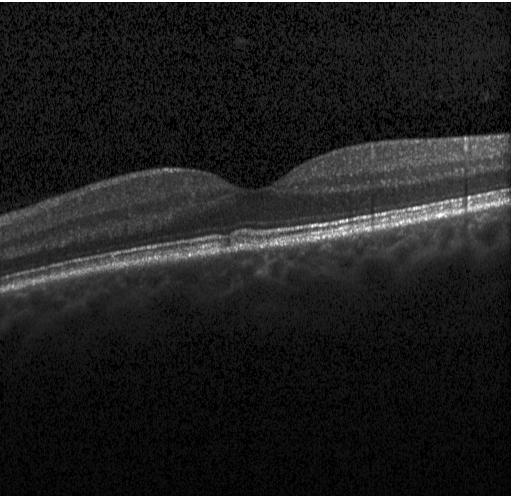
Acquired on a Heidelberg Spectralis, retinal OCT B-scan, macular scan, spectral-domain OCT — Impression: neither choroidal neovascularization, diabetic macular edema, nor drusen.